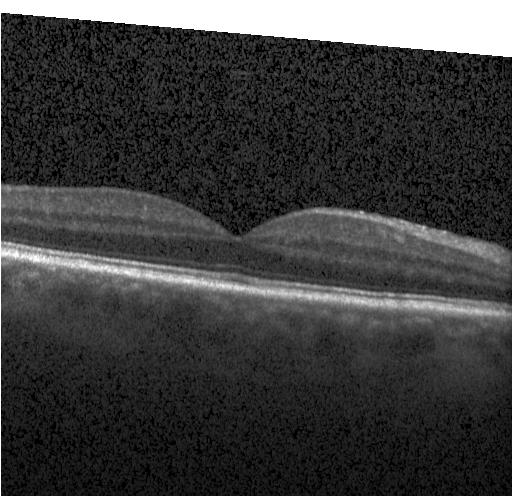
Retinal OCT cross-section, through the macula
Macular OCT: neither CNV, DME, nor drusen.